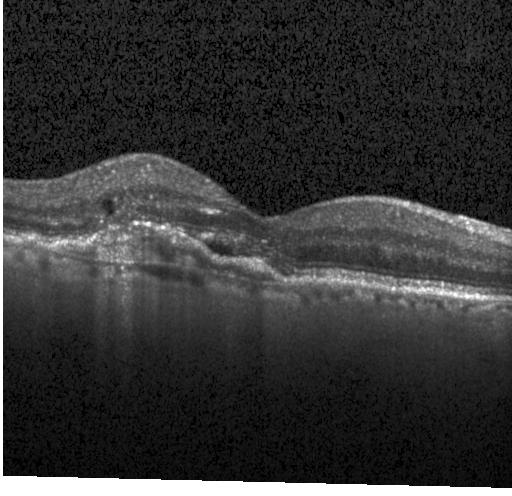

Macular OCT: choroidal neovascularization.